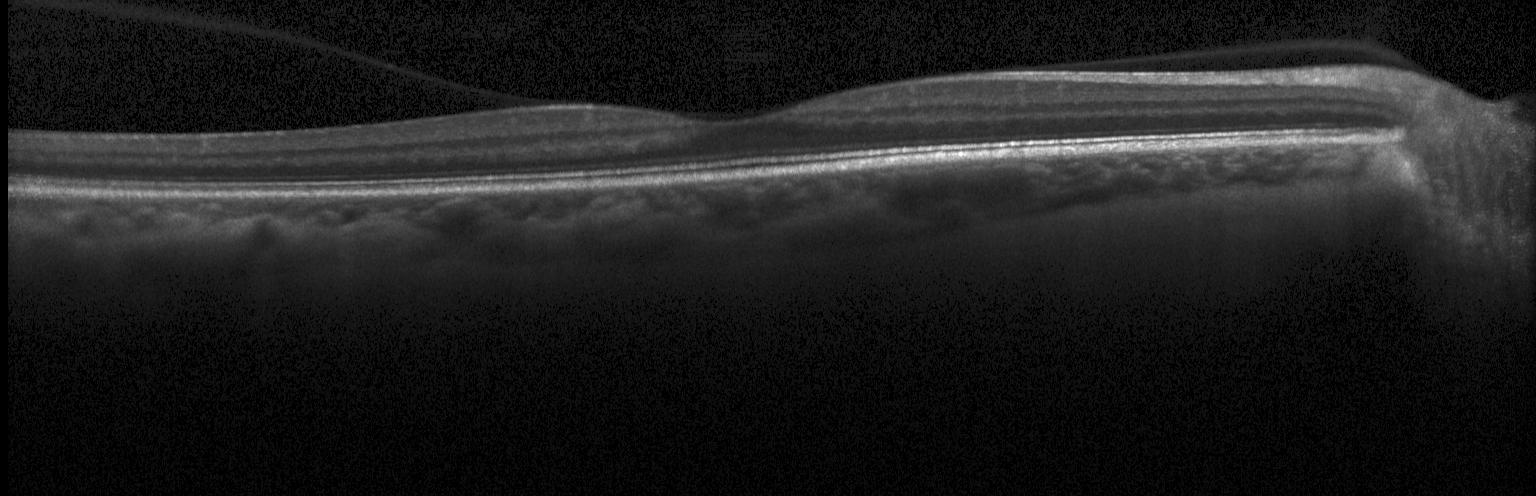

Diagnosis: neither CNV, DME, nor drusen.